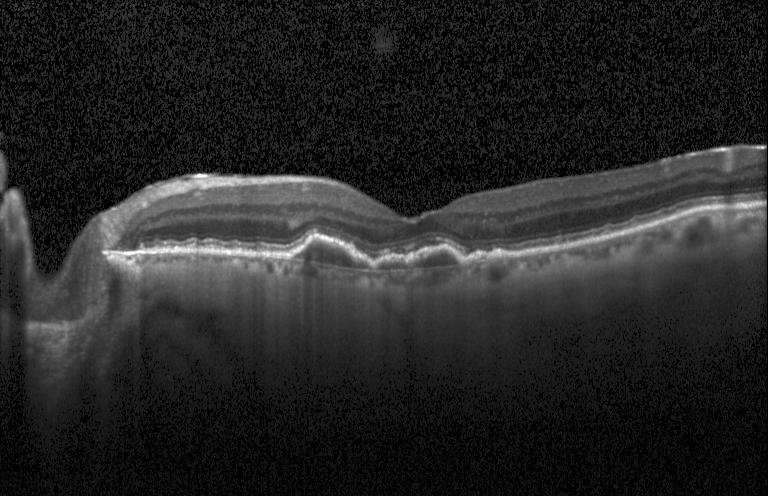 Spectral-domain optical coherence tomography, retinal OCT cross-section, through the macula, Heidelberg Spectralis. Diagnosis: a choroidal neovascular membrane.